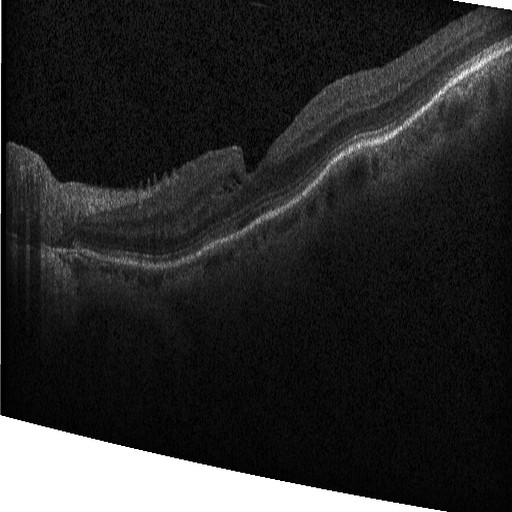

OCT line scan; Heidelberg Spectralis. Finding: DME.